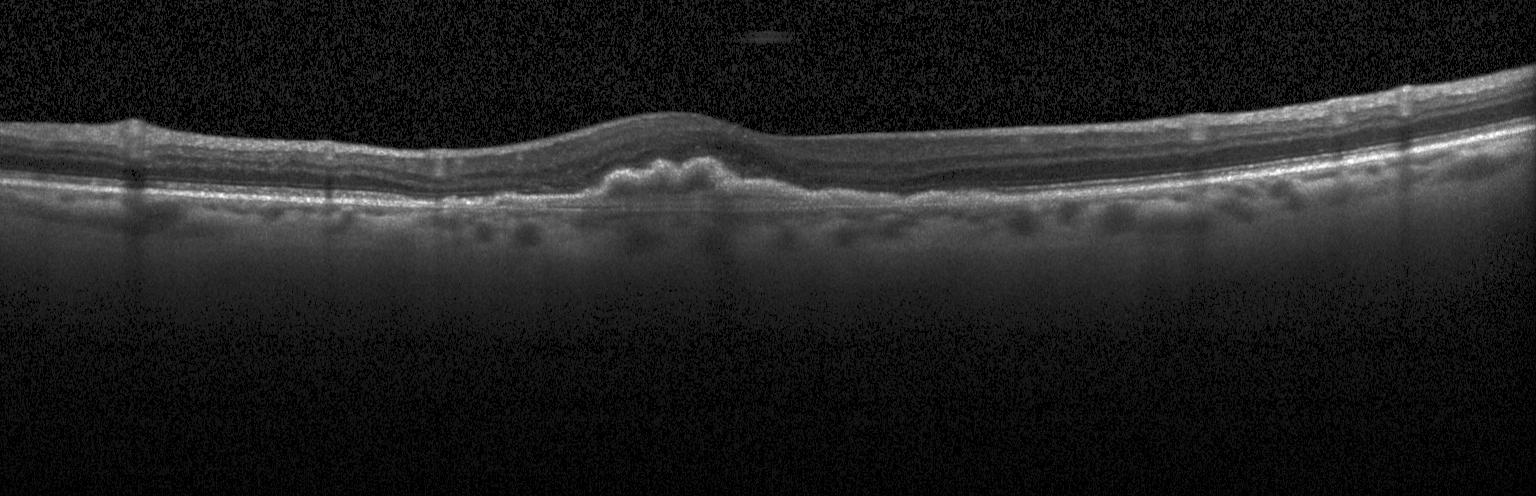 OCT B-scan showing a choroidal neovascular membrane.